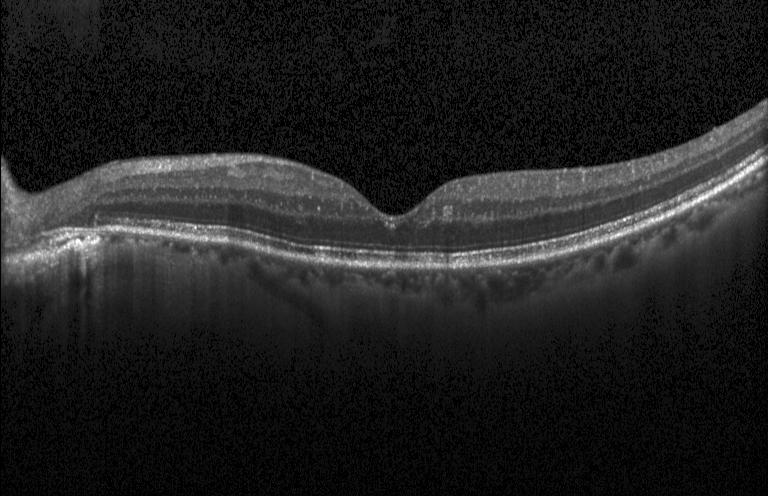 OCT finding: no choroidal neovascularization, no diabetic macular edema, and no drusen.